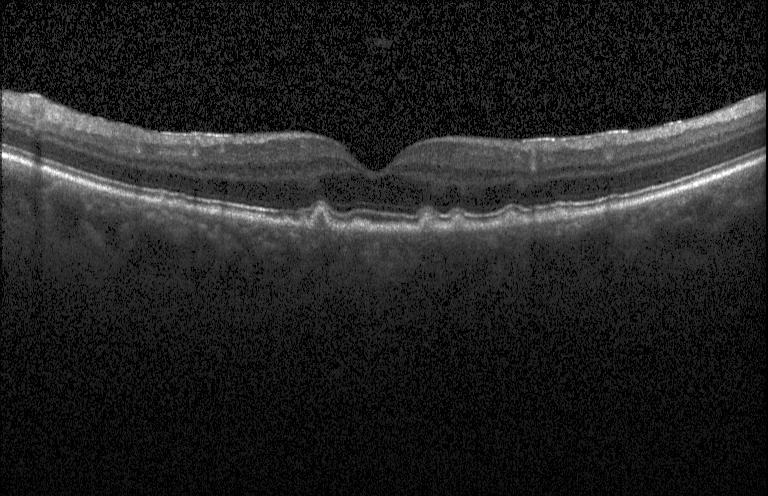 The scan shows sub-RPE drusenoid deposits.